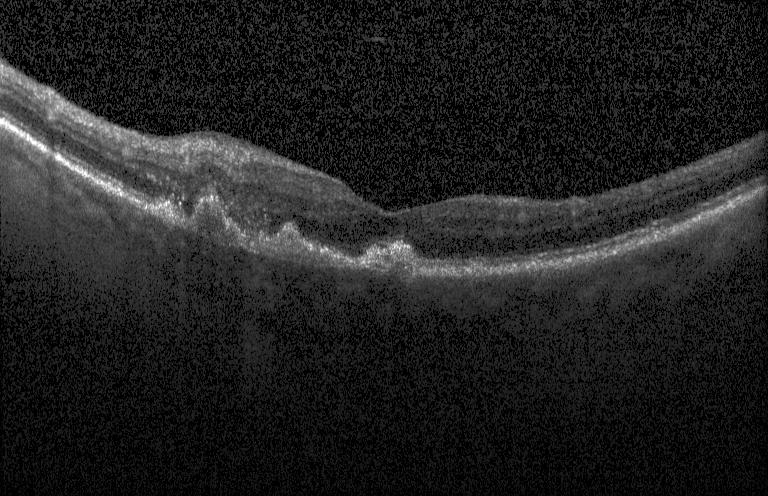
OCT line scan. Fovea-centered. Spectral-domain optical coherence tomography. Heidelberg Spectralis
Impression: CNV.